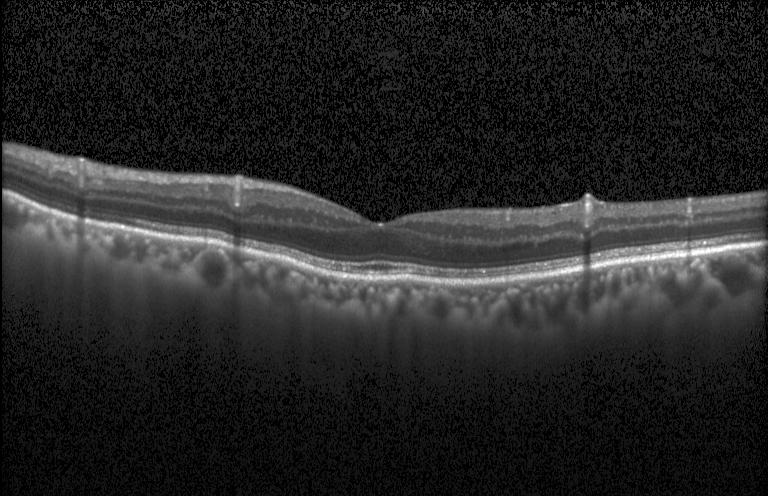 This B-scan demonstrates no choroidal neovascularization, no diabetic macular edema, and no drusen.